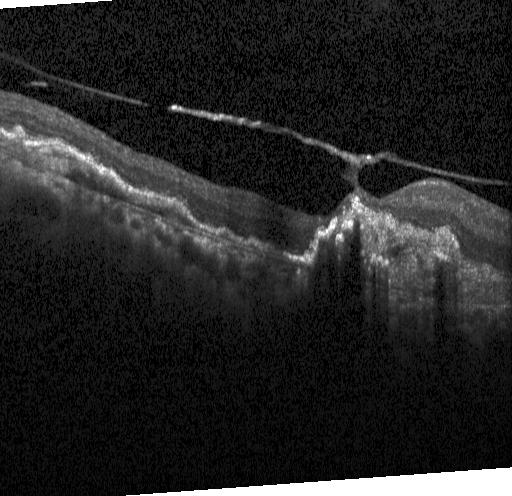
Fovea-centered. Optical coherence tomography scan. Instrument: Heidelberg Spectralis
Choroidal neovascularization.